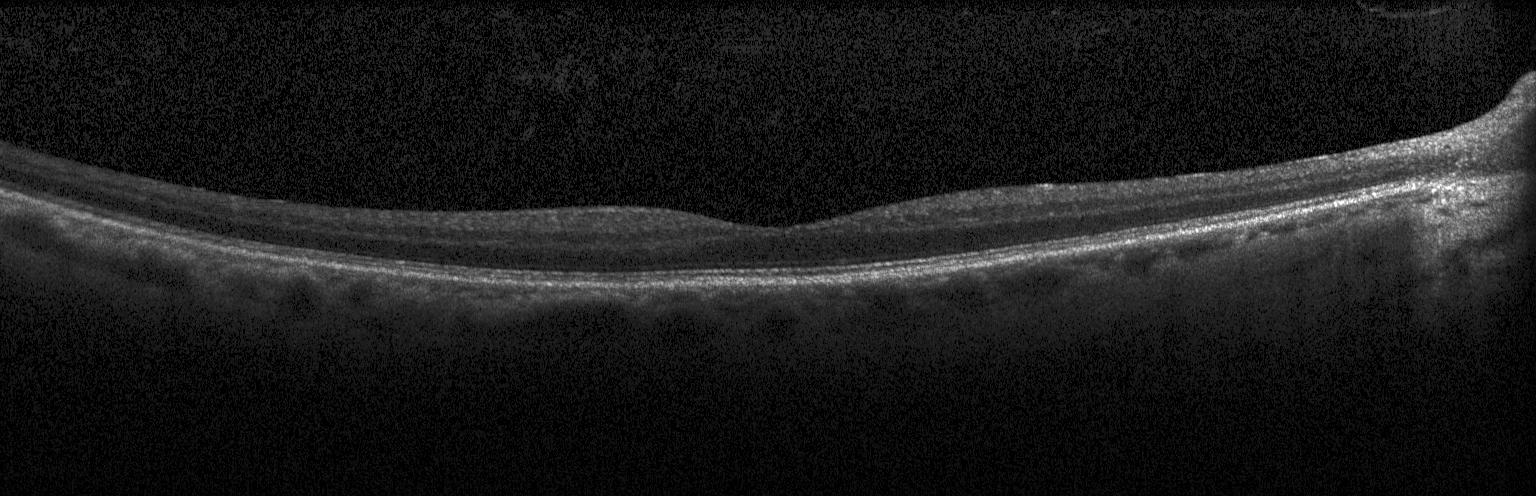 Retinal OCT cross-section
Neither CNV, DME, nor drusen.